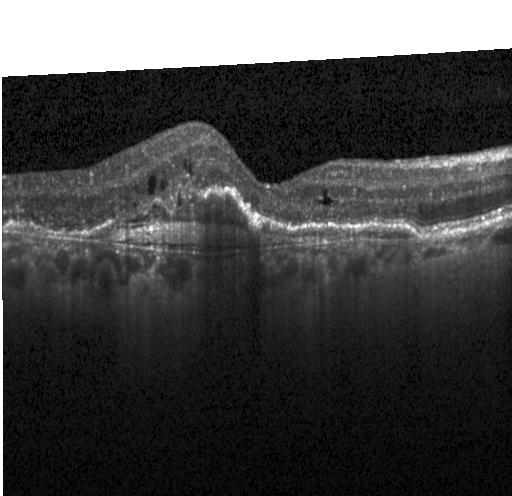 Macular OCT demonstrating CNV.